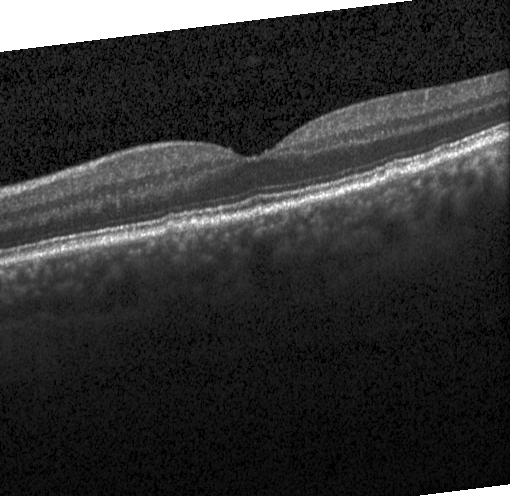

Heidelberg Spectralis OCT system; spectral-domain optical coherence tomography; retinal OCT cross-section.
Finding: drusen.